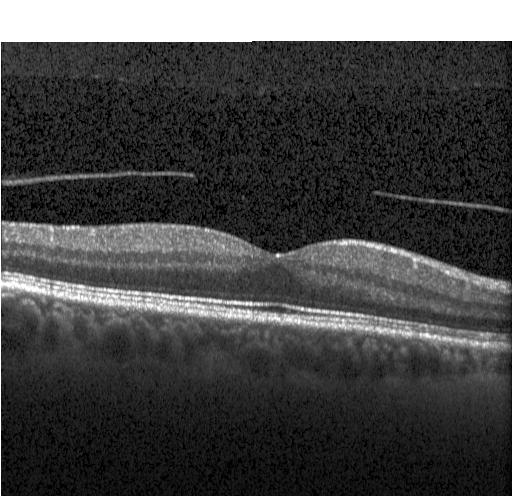 OCT B-scan, through the macula. Finding: no evidence of choroidal neovascularization, diabetic macular edema, or drusen.